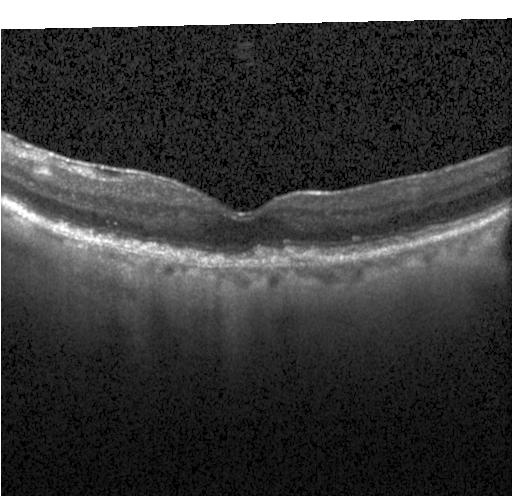
Diagnosis: sub-RPE drusenoid deposits.